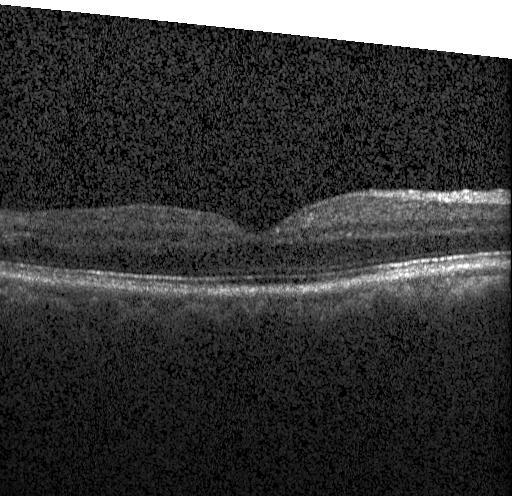

Retinal OCT cross-section showing neither choroidal neovascularization, diabetic macular edema, nor drusen.